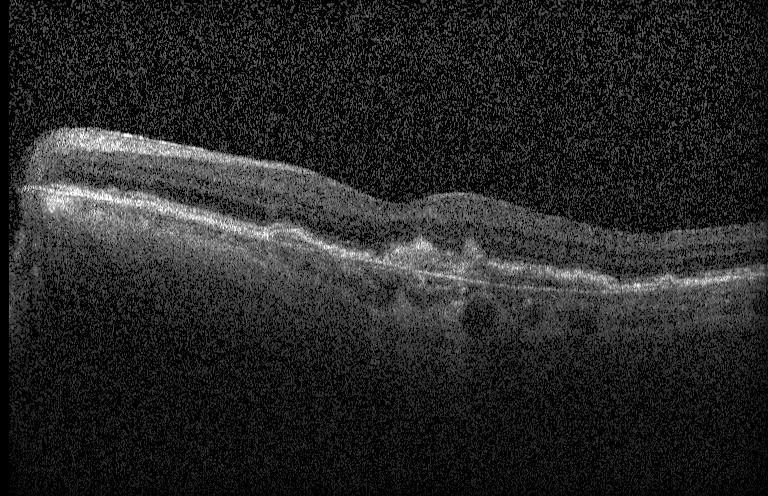
Retinal OCT cross-section · fovea-centered · Heidelberg Spectralis OCT system.
Impression: a choroidal neovascular membrane.